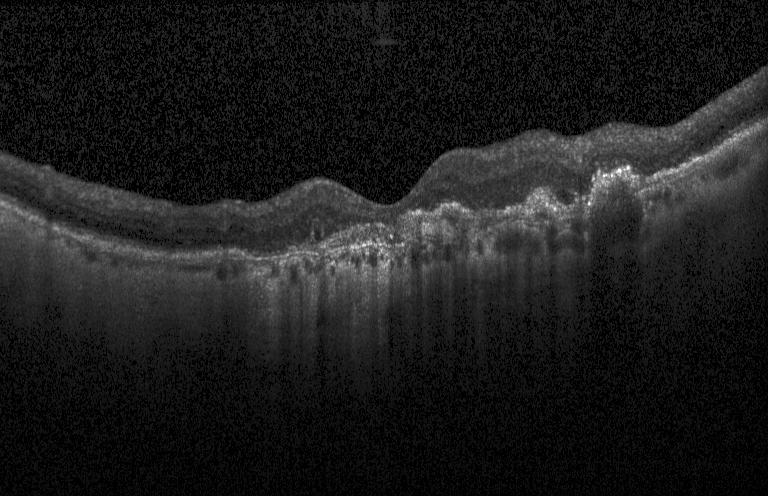

Fovea-centered; OCT B-scan; instrument: Heidelberg Spectralis
Finding: choroidal neovascularization.